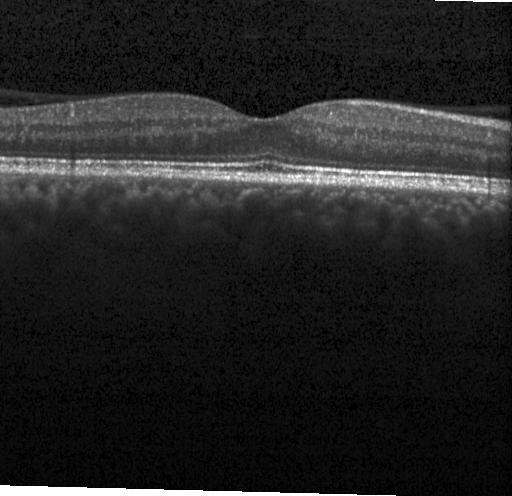 Macular OCT: no choroidal neovascularization, no diabetic macular edema, and no drusen.